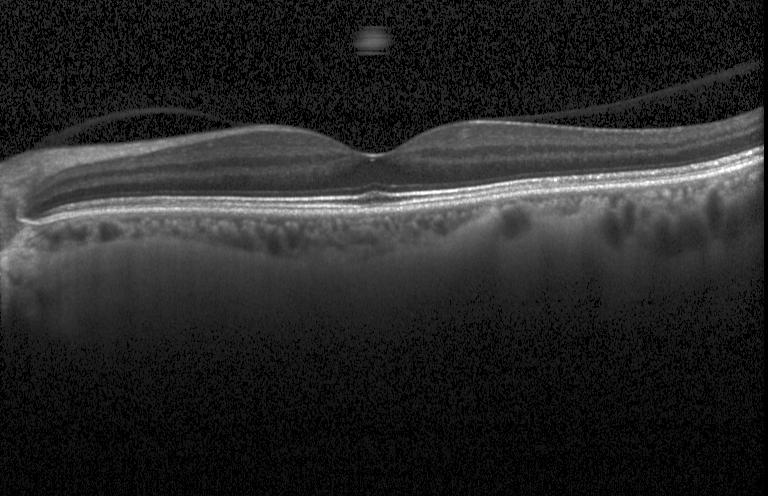

Instrument: Heidelberg Spectralis · retinal OCT B-scan · centered on the fovea. Dx: neither choroidal neovascularization, diabetic macular edema, nor drusen.